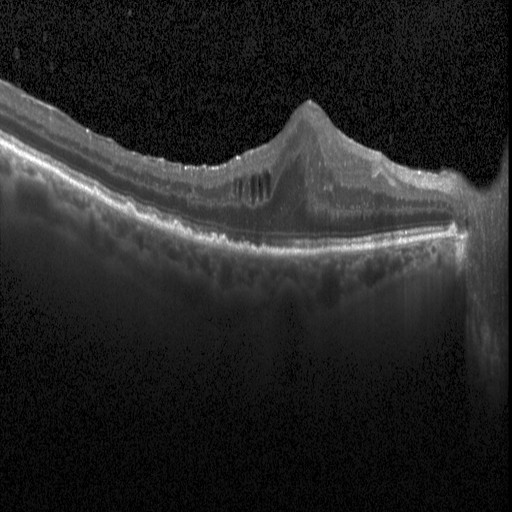

Optical coherence tomography scan, spectral-domain OCT
Diagnosis: DME.